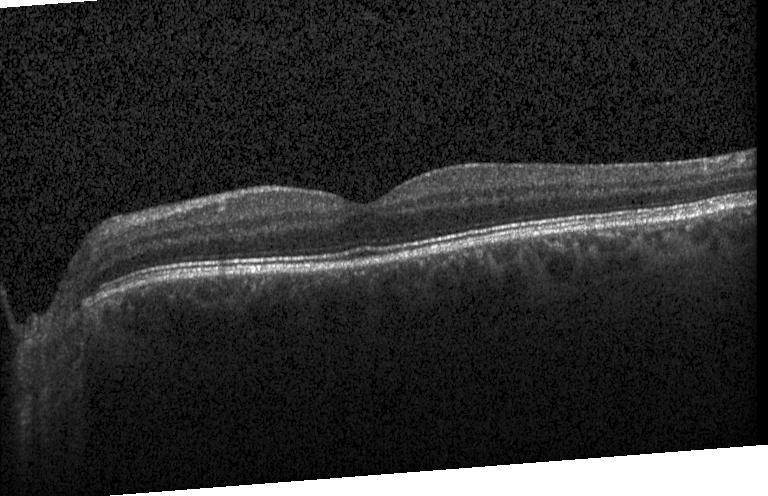
Spectral-domain optical coherence tomography · OCT B-scan · macular scan.
Impression: no evidence of choroidal neovascularization, diabetic macular edema, or drusen.